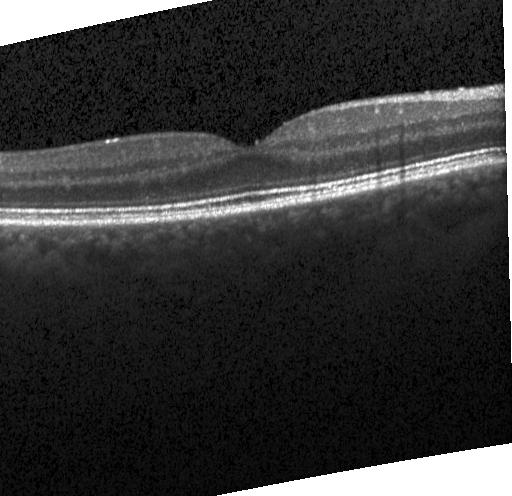

OCT B-scan; instrument: Heidelberg Spectralis
The scan shows no choroidal neovascularization, diabetic macular edema, or drusen.